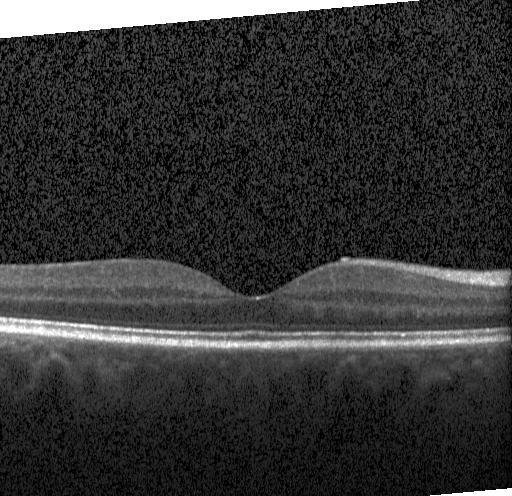 Macular OCT: no choroidal neovascularization, diabetic macular edema, or drusen.